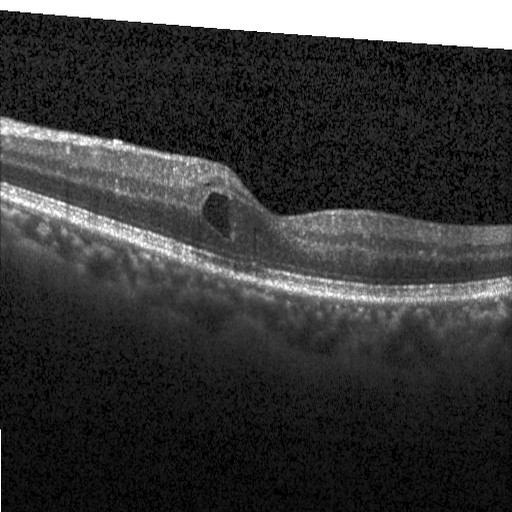
OCT line scan — Dx: DME.